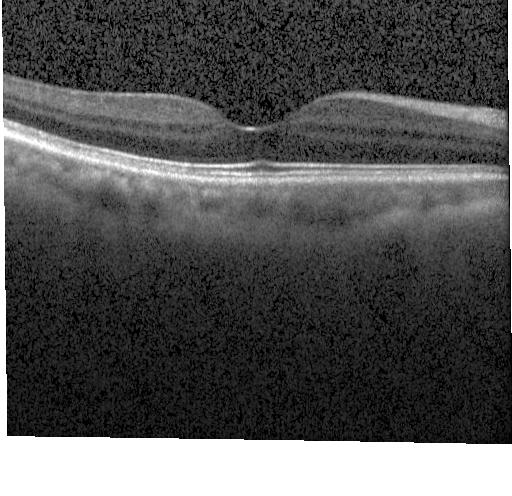
Dx: no CNV, DME, or drusen.